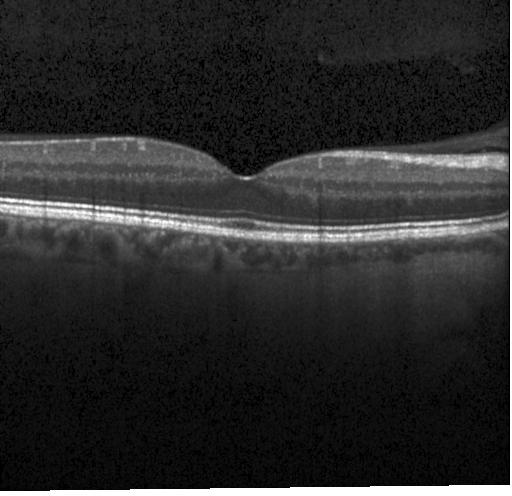 Retinal OCT cross-section. Spectral-domain OCT — Dx: no evidence of CNV, DME, or drusen.